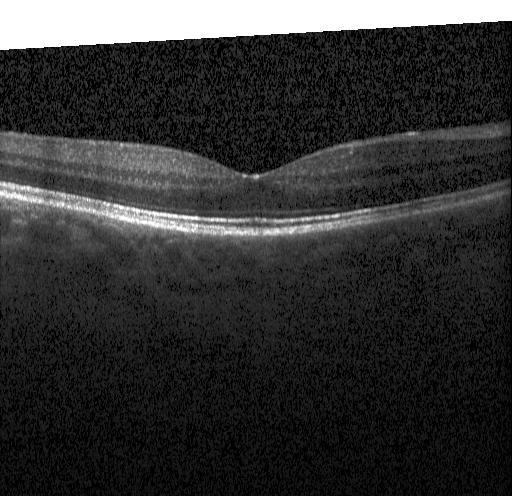 No CNV, no DME, and no drusen.